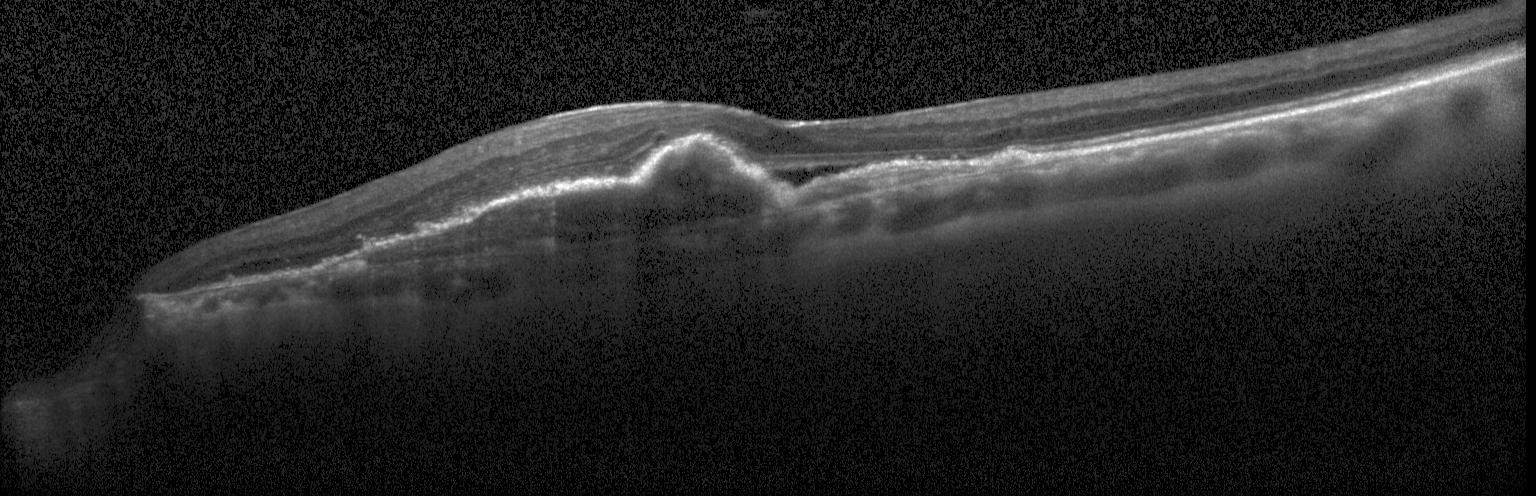
Spectral-domain optical coherence tomography; macular scan; OCT line scan; Heidelberg Spectralis OCT system.
This B-scan demonstrates choroidal neovascularization.